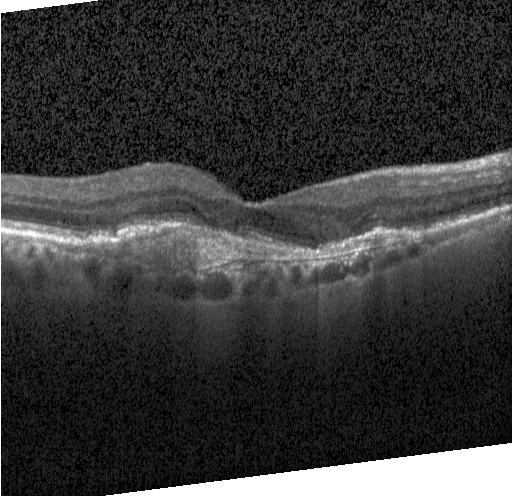
Diagnosis: CNV.